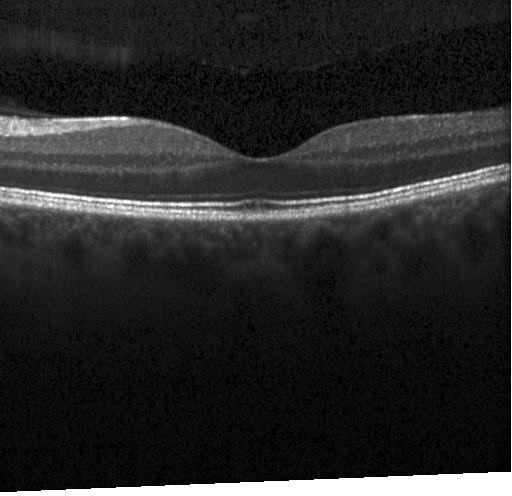 OCT finding: no choroidal neovascularization, no diabetic macular edema, and no drusen.